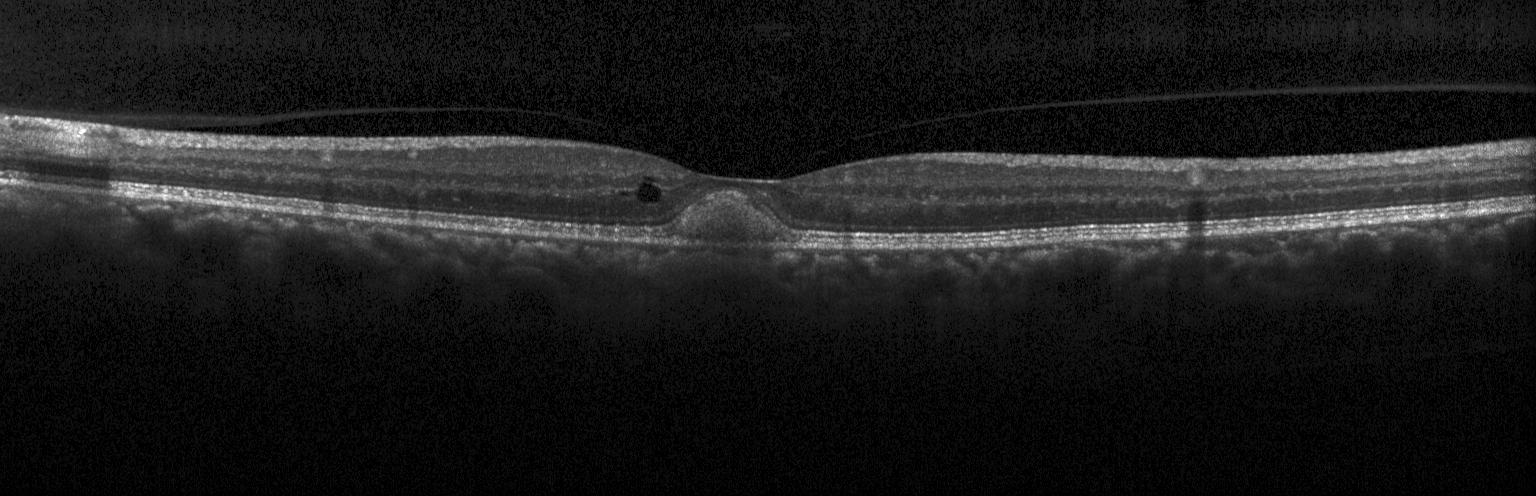
Heidelberg Spectralis OCT system. Retinal OCT cross-section — Diagnosis: CNV.